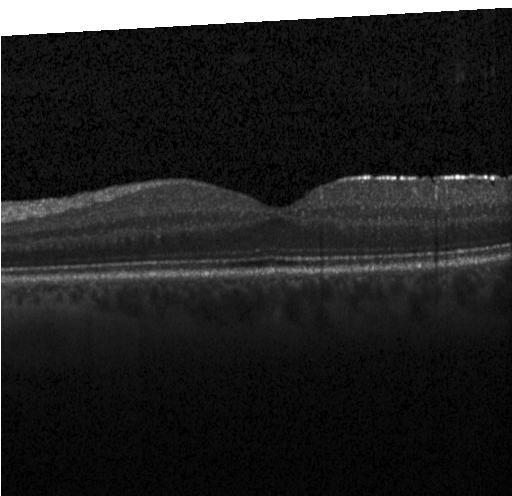
OCT finding: neither choroidal neovascularization, diabetic macular edema, nor drusen.